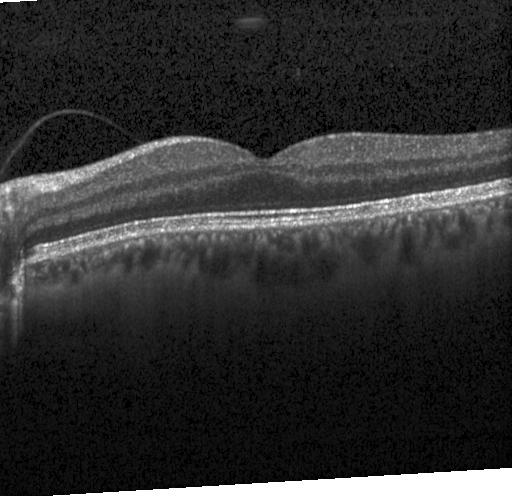
OCT finding: no CNV, DME, or drusen.